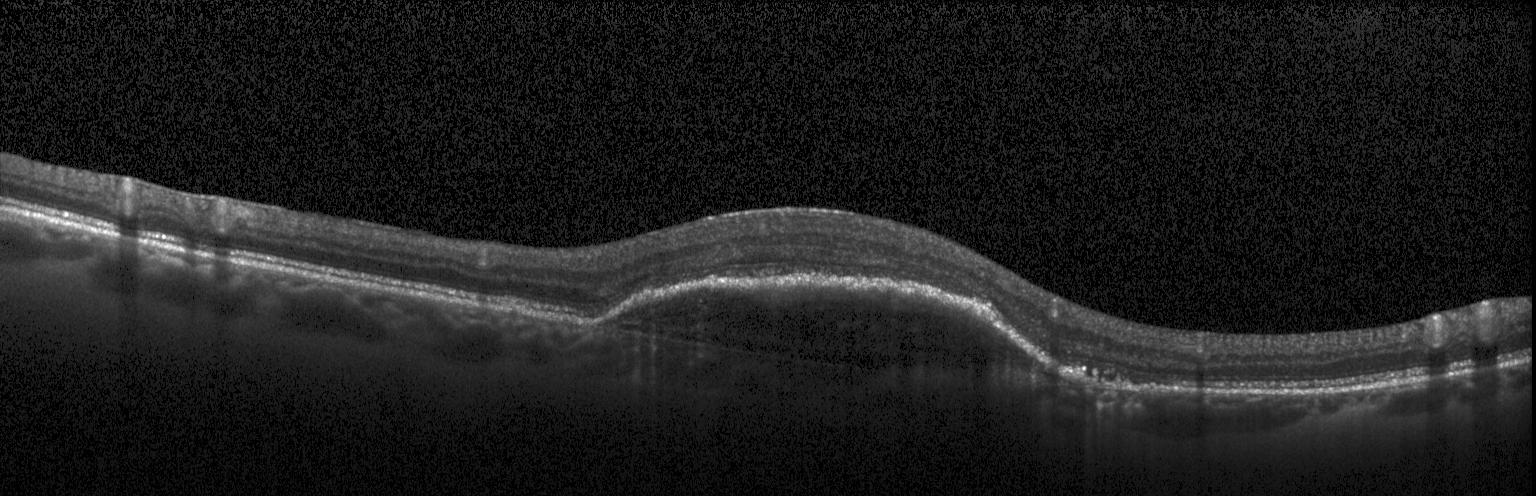 Diagnosis: a choroidal neovascular membrane.